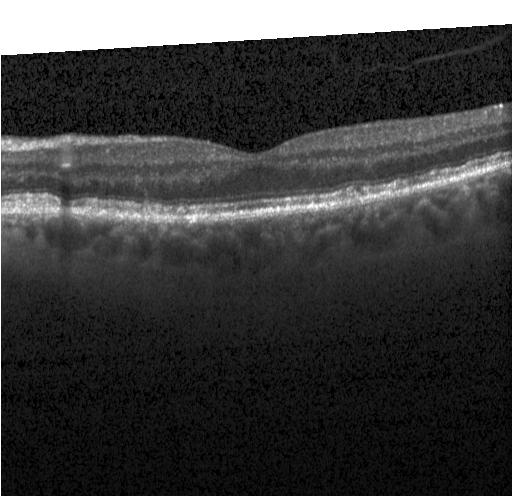
This B-scan demonstrates sub-RPE drusenoid deposits.